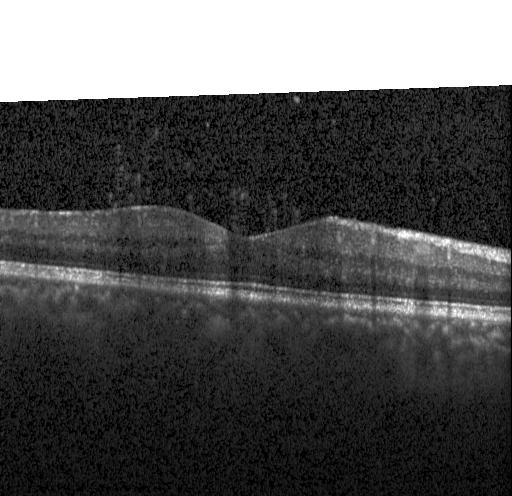
Spectral-domain OCT, fovea-centered, optical coherence tomography scan, Heidelberg Spectralis — Macular OCT: no CNV, DME, or drusen.